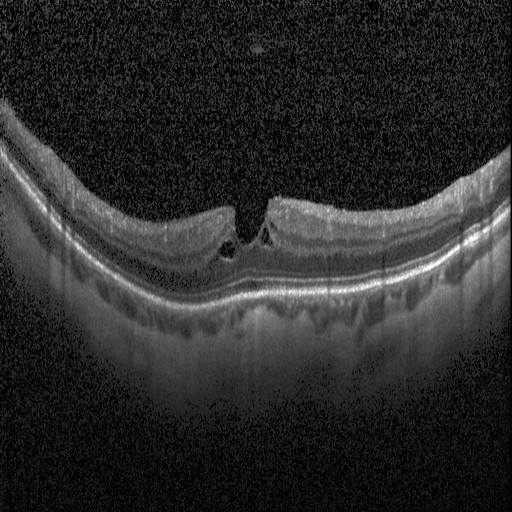

OCT B-scan — This B-scan demonstrates diabetic macular edema.